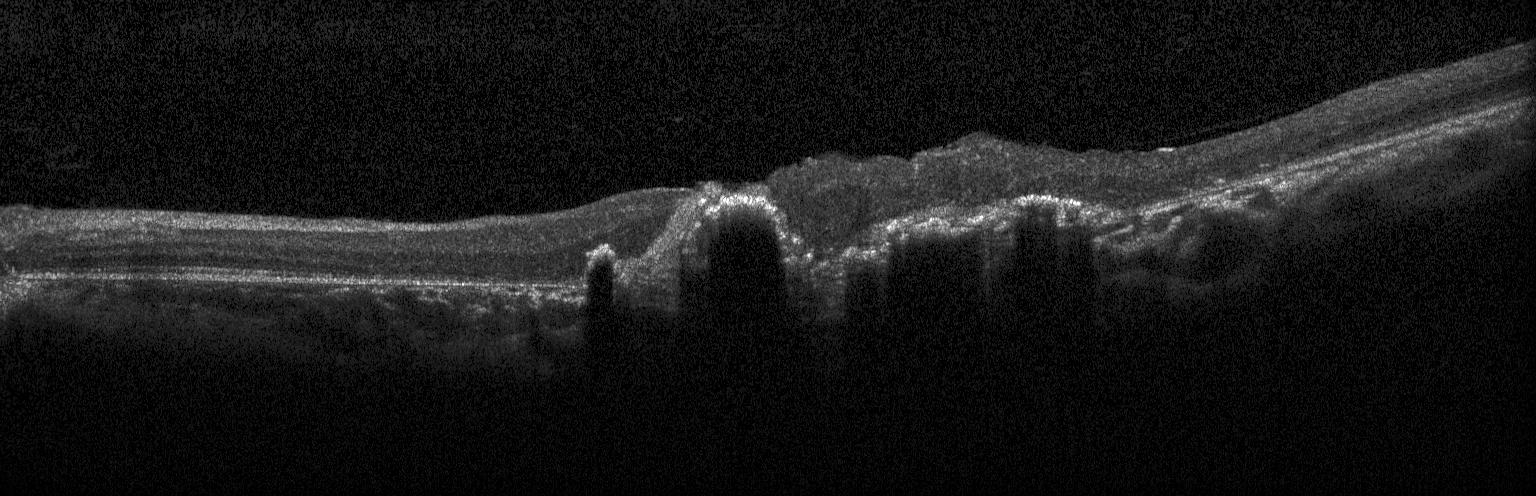

OCT B-scan. Dx: choroidal neovascularization (CNV).